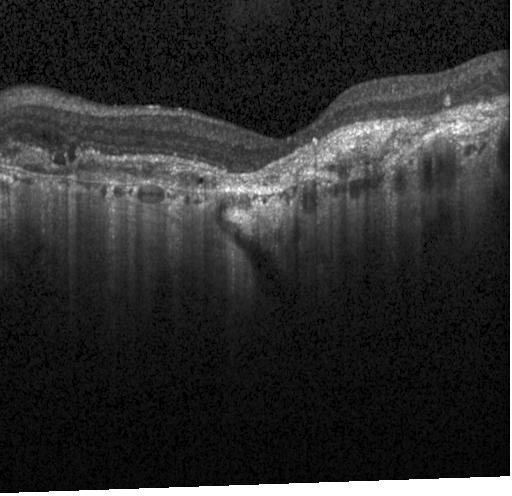 OCT line scan; Heidelberg Spectralis OCT system — Finding: a choroidal neovascular membrane.